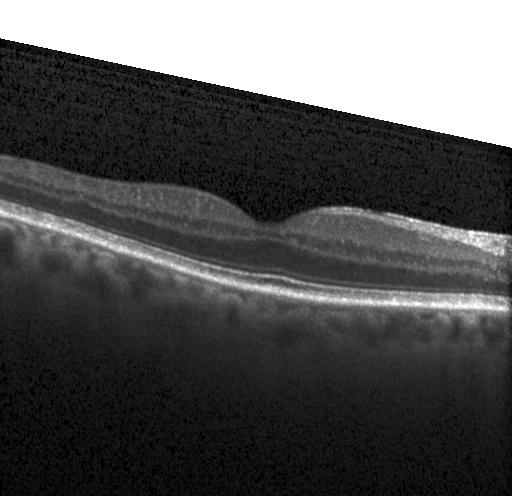
Spectral-domain OCT. Optical coherence tomography scan
Impression: neither choroidal neovascularization, diabetic macular edema, nor drusen.